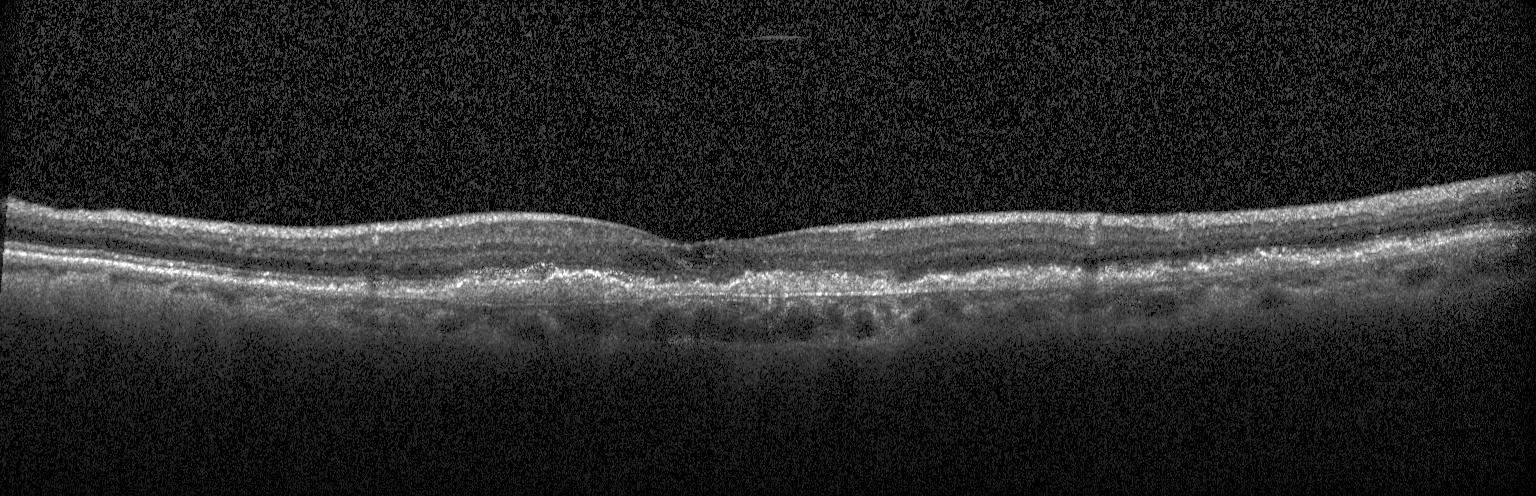

Heidelberg Spectralis OCT system · optical coherence tomography B-scan · through the macula — Diagnosis: choroidal neovascularization.